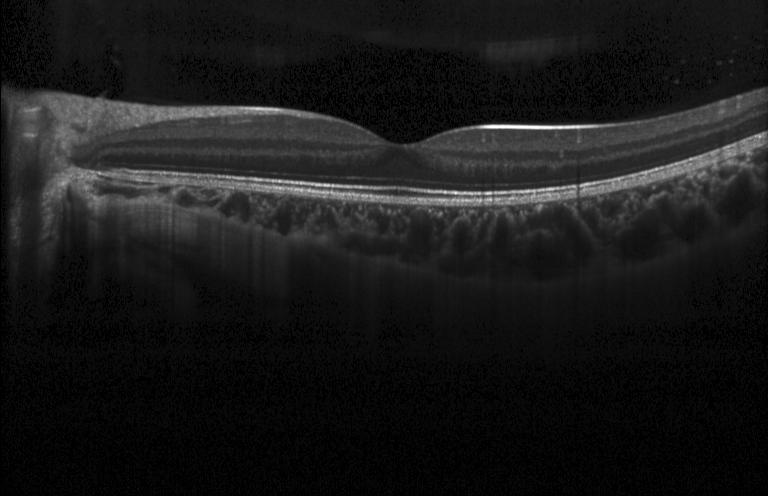
Finding: no evidence of CNV, DME, or drusen.